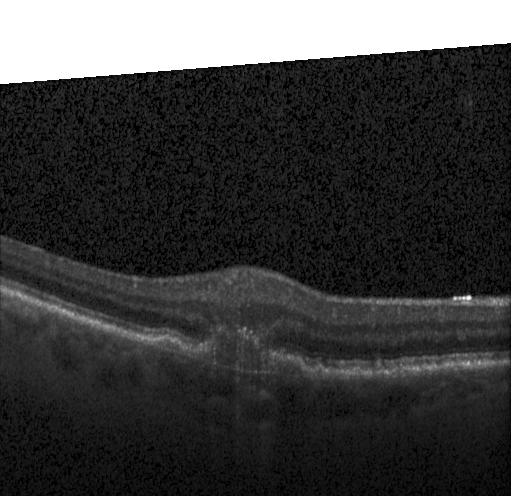 Heidelberg Spectralis, optical coherence tomography scan, spectral-domain OCT, fovea-centered — The scan shows choroidal neovascularization (CNV).